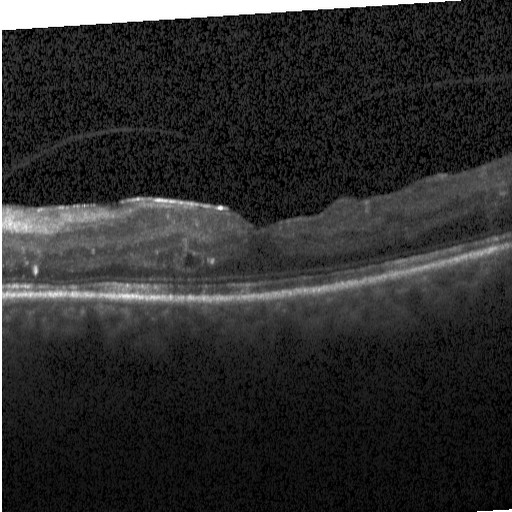 Optical coherence tomography scan.
This B-scan demonstrates DME.